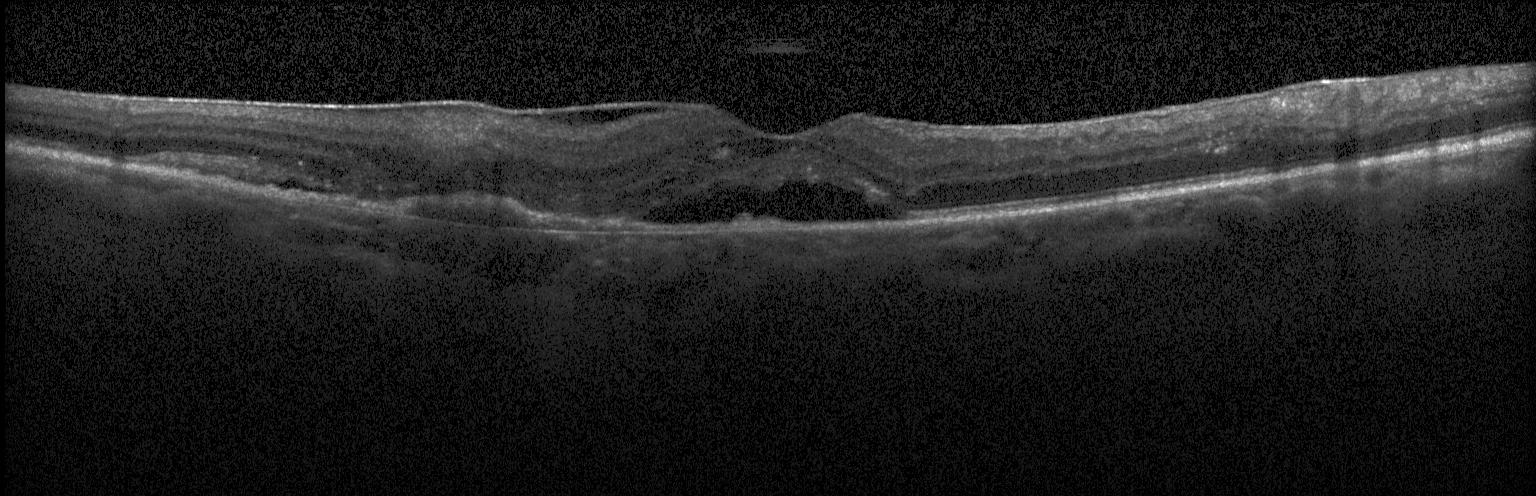
Diagnosis: a choroidal neovascular membrane.